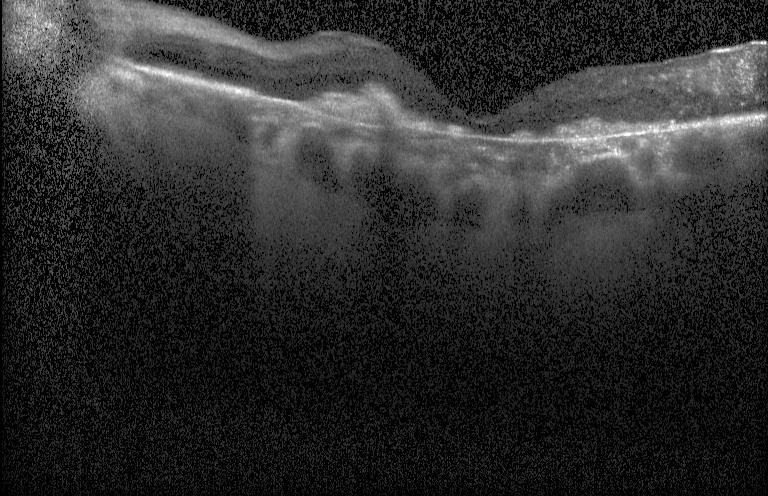
Macular OCT: choroidal neovascularization (CNV).